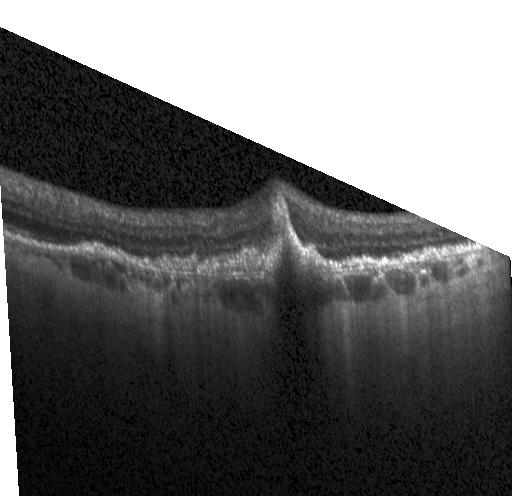

Acquired on a Heidelberg Spectralis. OCT B-scan
OCT finding: a choroidal neovascular membrane.